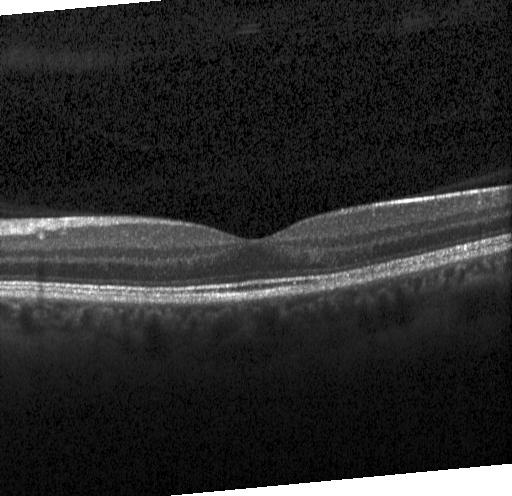

OCT B-scan showing neither CNV, DME, nor drusen.